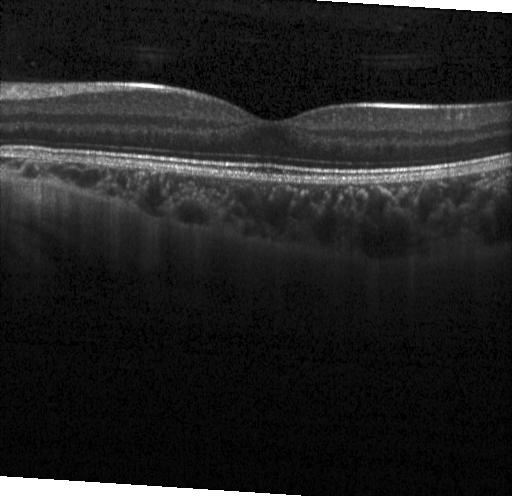 Macular OCT: neither choroidal neovascularization, diabetic macular edema, nor drusen.